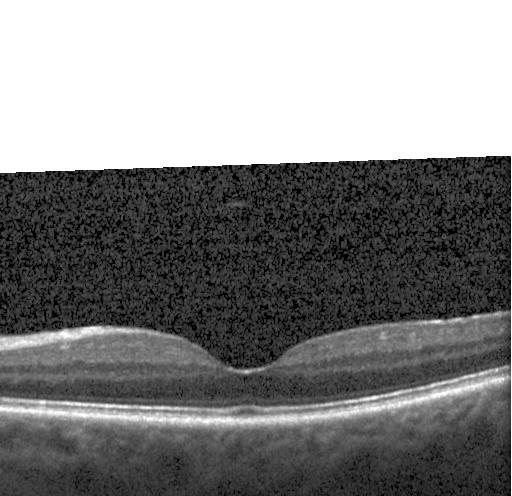
Heidelberg Spectralis. OCT line scan. Spectral-domain OCT. Centered on the fovea
Impression: no choroidal neovascularization, no diabetic macular edema, and no drusen.